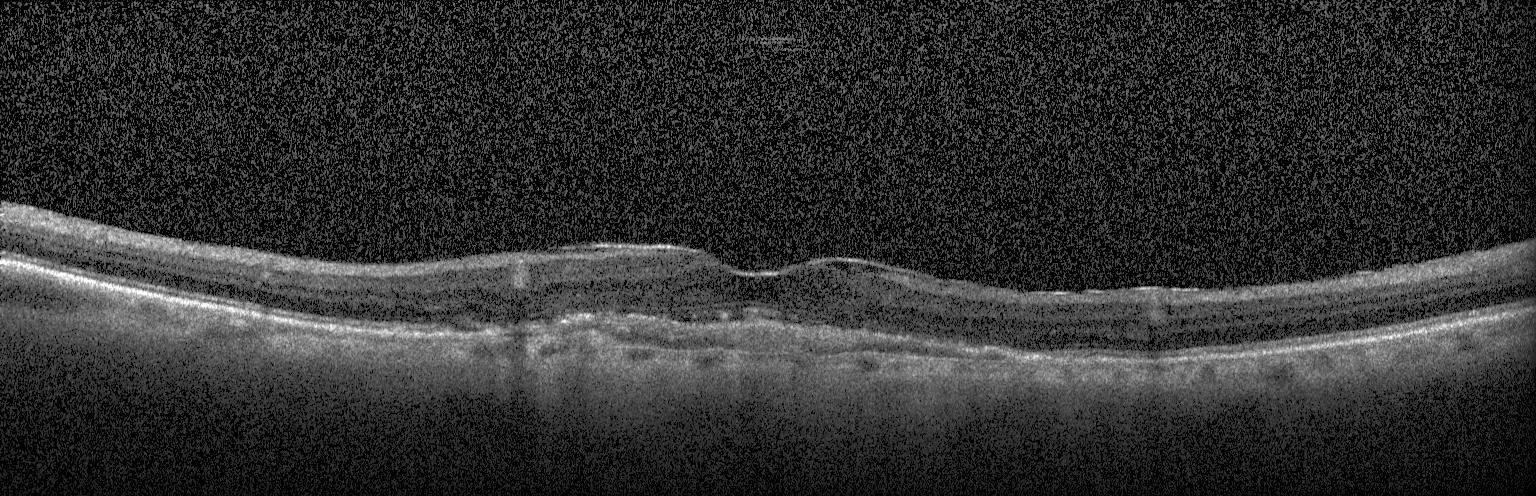

Retinal OCT B-scan · SD-OCT · centered on the fovea. Impression: CNV.